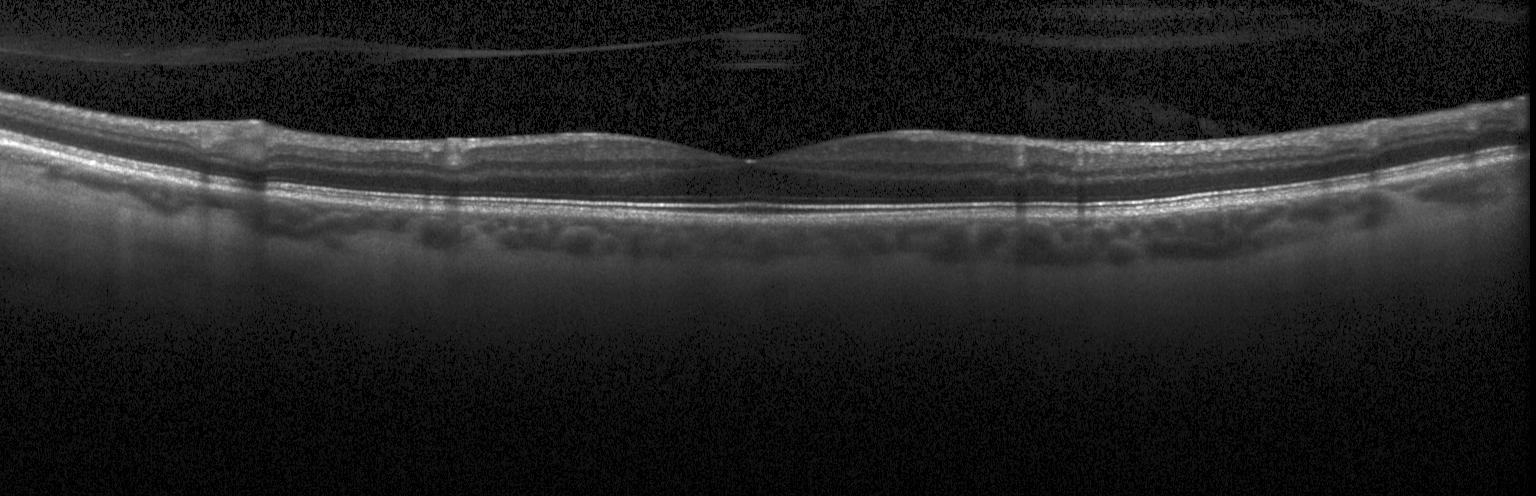

Retinal OCT B-scan; fovea-centered; SD-OCT — This B-scan demonstrates neither choroidal neovascularization, diabetic macular edema, nor drusen.